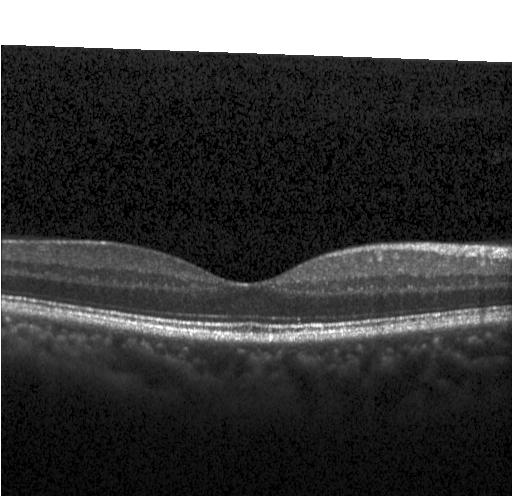 OCT finding: neither CNV, DME, nor drusen.